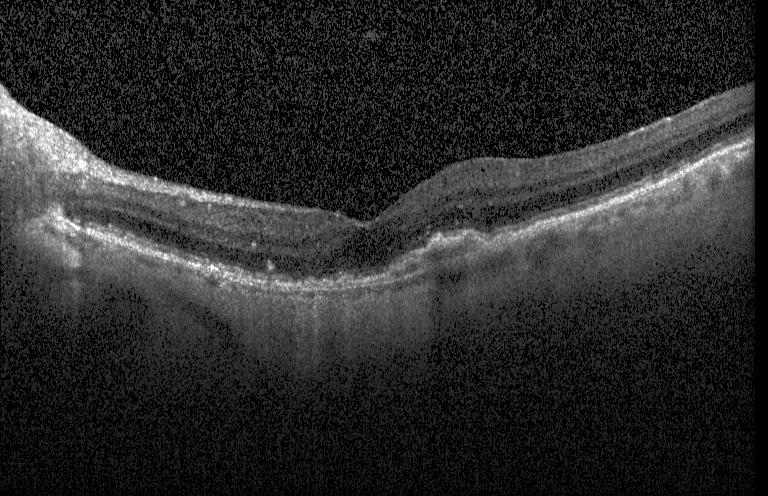 Heidelberg Spectralis OCT system · optical coherence tomography scan. Assessment: a choroidal neovascular membrane.